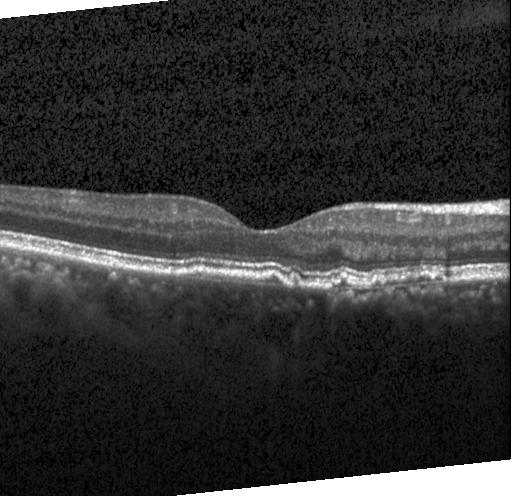 Optical coherence tomography scan · horizontal scan through the fovea · spectral-domain optical coherence tomography · Heidelberg Spectralis OCT system
Assessment: drusen.